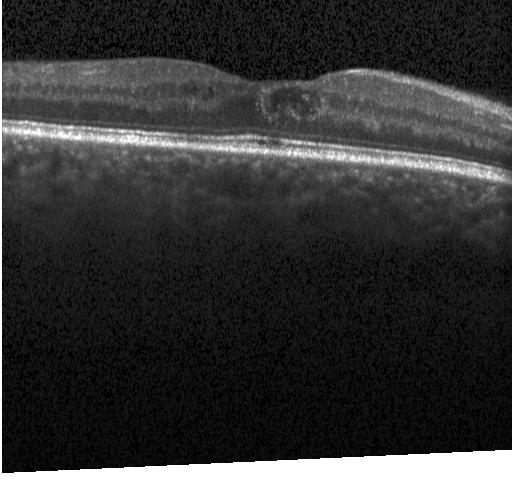

Heidelberg Spectralis, spectral-domain optical coherence tomography, retinal OCT B-scan. Impression: diabetic macular edema (DME).